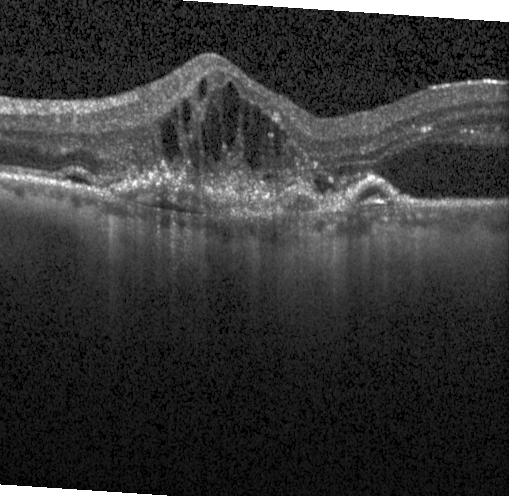

OCT finding: a choroidal neovascular membrane.